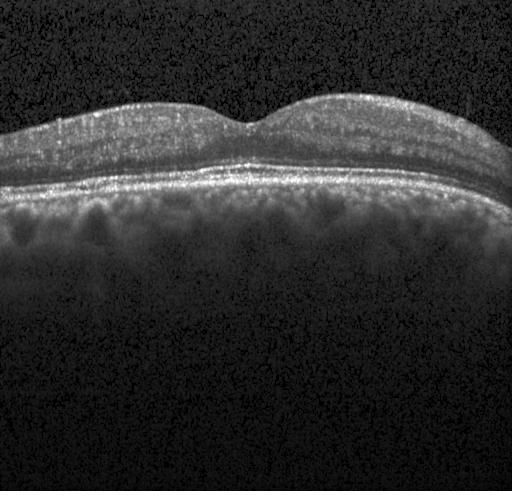

OCT line scan — Assessment: no choroidal neovascularization, diabetic macular edema, or drusen.